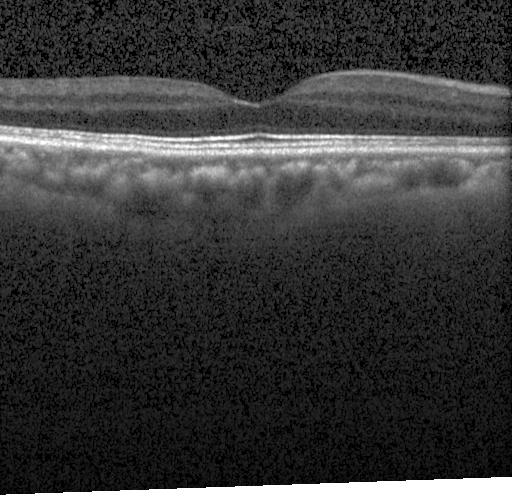

Horizontal scan through the fovea. SD-OCT. Retinal OCT cross-section
Diagnosis: neither choroidal neovascularization, diabetic macular edema, nor drusen.